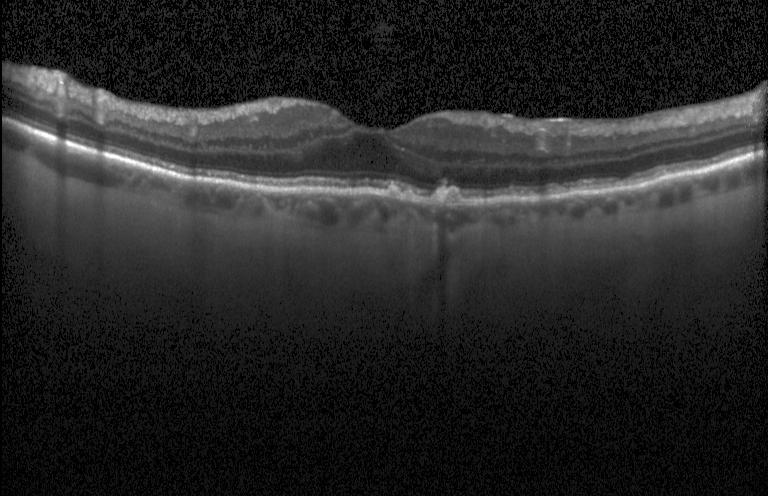 OCT line scan — Impression: drusen.